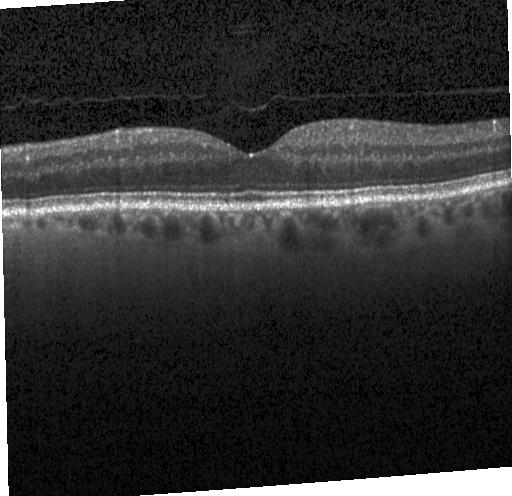 Retinal OCT cross-section.
No CNV, DME, or drusen.